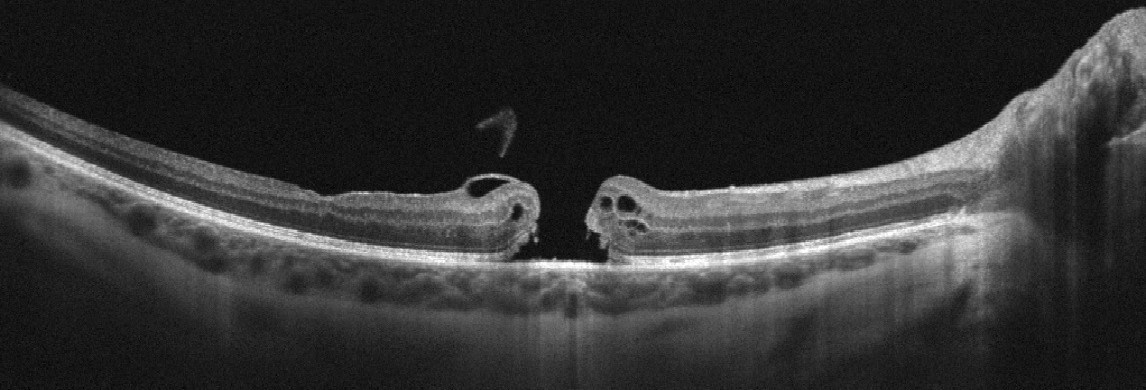

Retinal OCT cross-section; macular scan.
Impression: vitreomacular interface disease (VID).